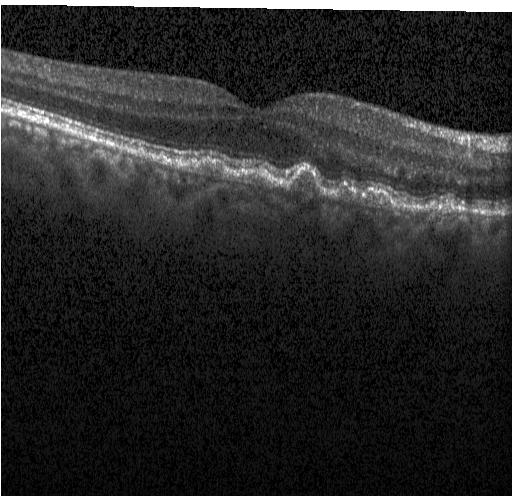 Diagnosis: multiple drusen.